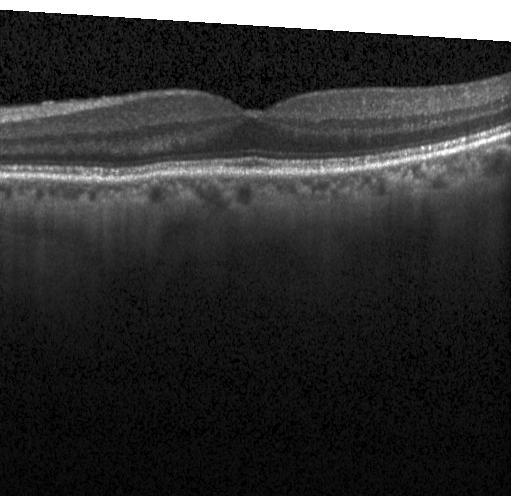

OCT finding: no evidence of choroidal neovascularization, diabetic macular edema, or drusen.